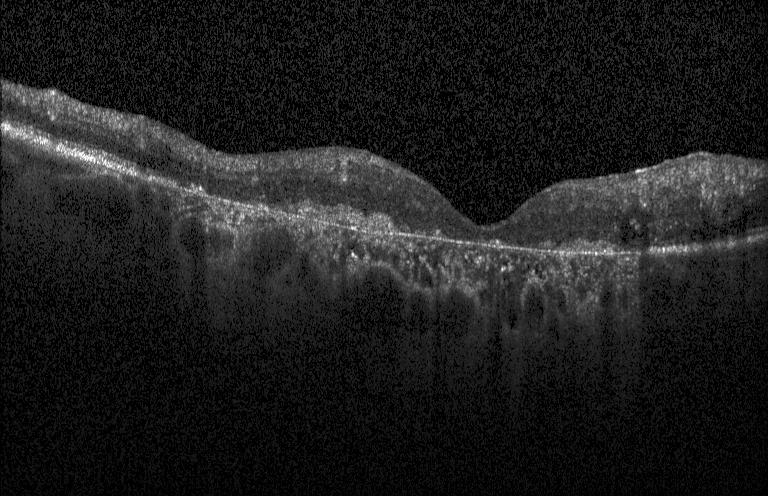 Macular scan. Optical coherence tomography B-scan. Acquired on a Heidelberg Spectralis. Spectral-domain OCT
Diagnosis: CNV.